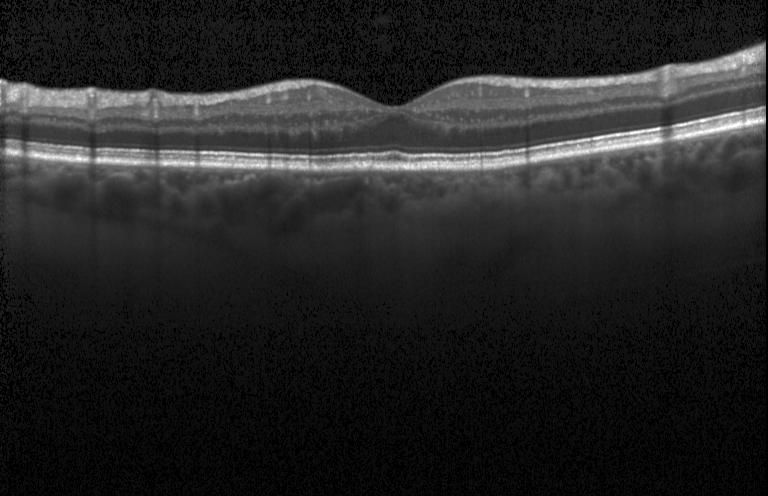 Diagnosis: no CNV, no DME, and no drusen.